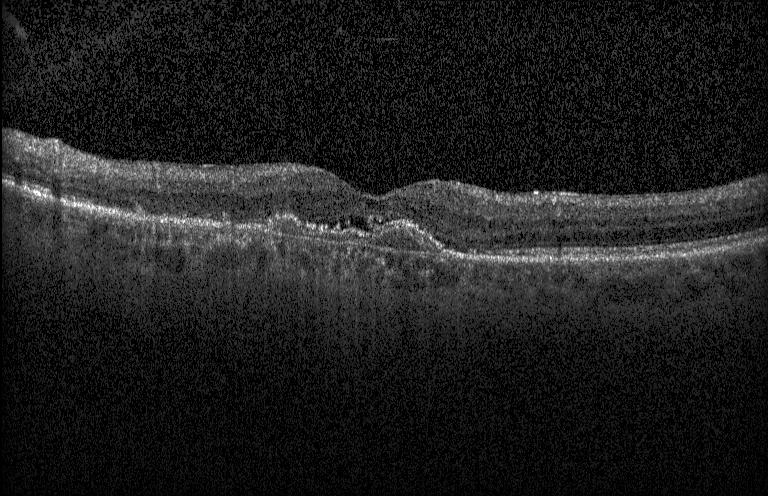
Impression: a choroidal neovascular membrane.